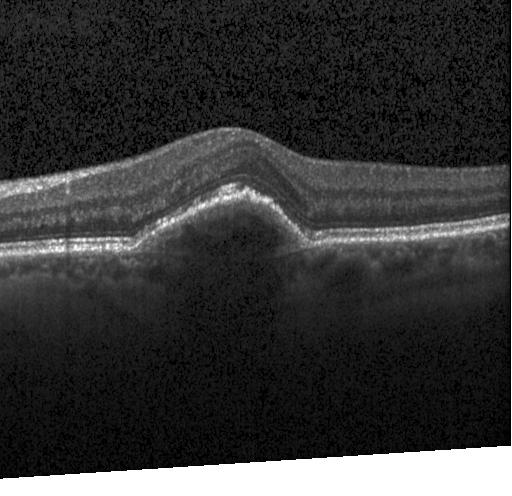
SD-OCT · fovea-centered · retinal OCT cross-section · acquired on a Heidelberg Spectralis
Finding: a choroidal neovascular membrane.